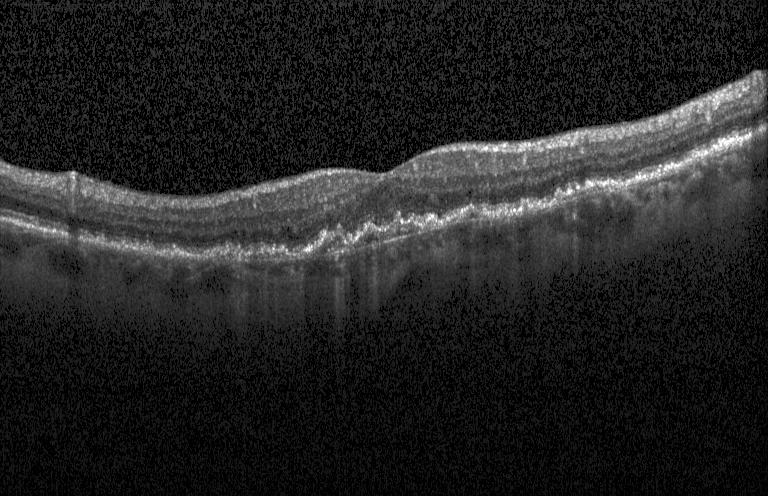 Assessment: choroidal neovascularization.